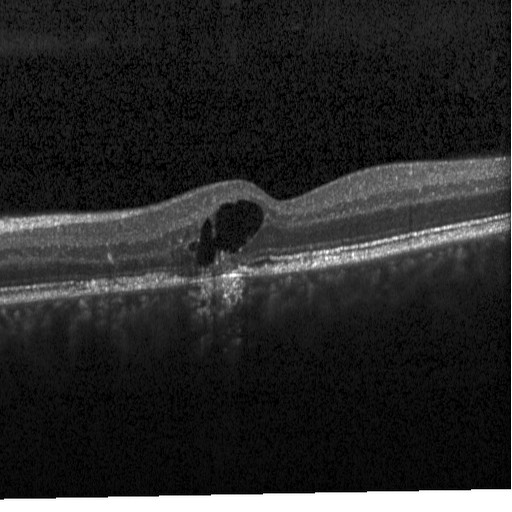
Diagnosis: DME.